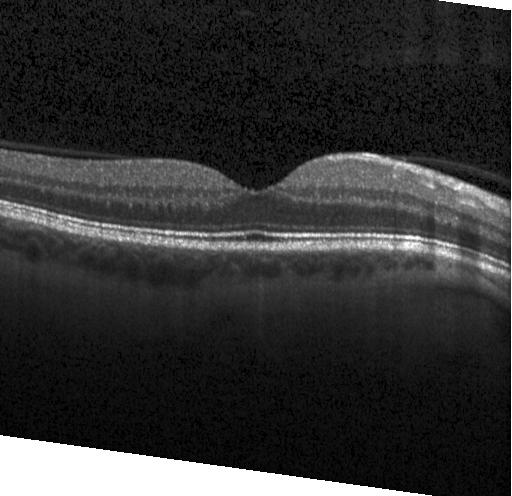
Spectral-domain OCT B-scan: no choroidal neovascularization, diabetic macular edema, or drusen.